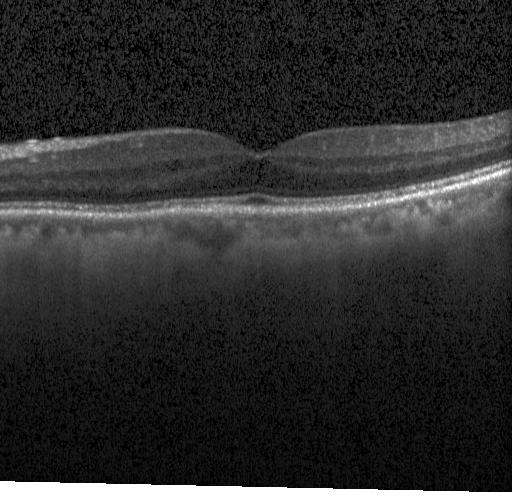 OCT B-scan. Diagnosis: no choroidal neovascularization, diabetic macular edema, or drusen.